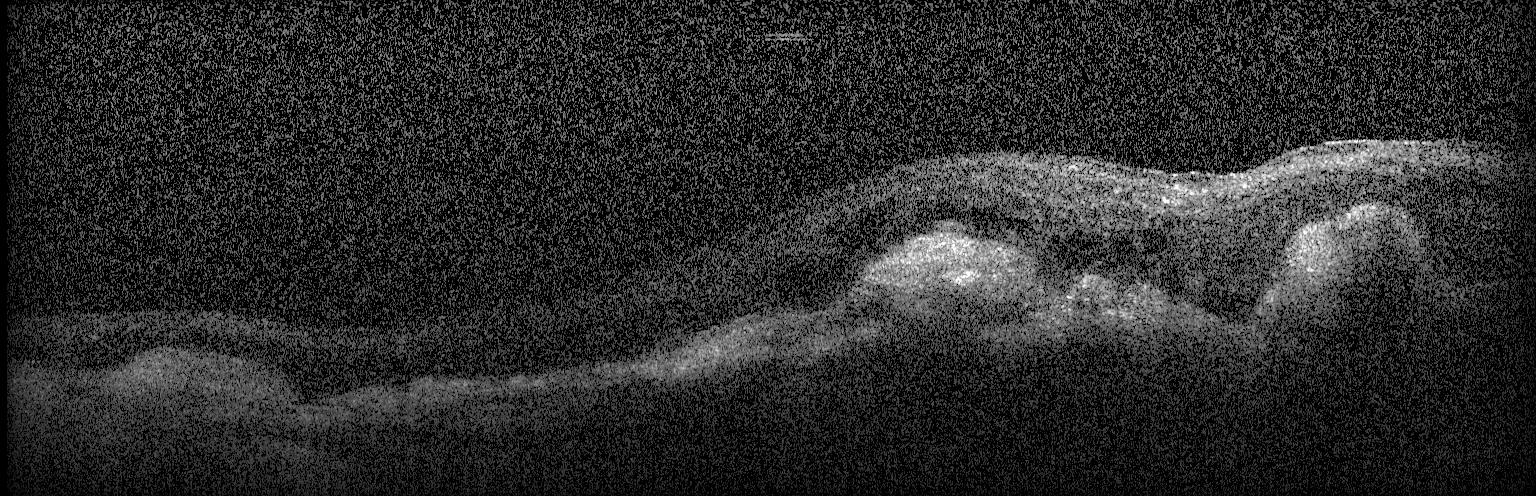
Instrument: Heidelberg Spectralis; centered on the fovea; optical coherence tomography scan; spectral-domain OCT — Finding: choroidal neovascularization (CNV).